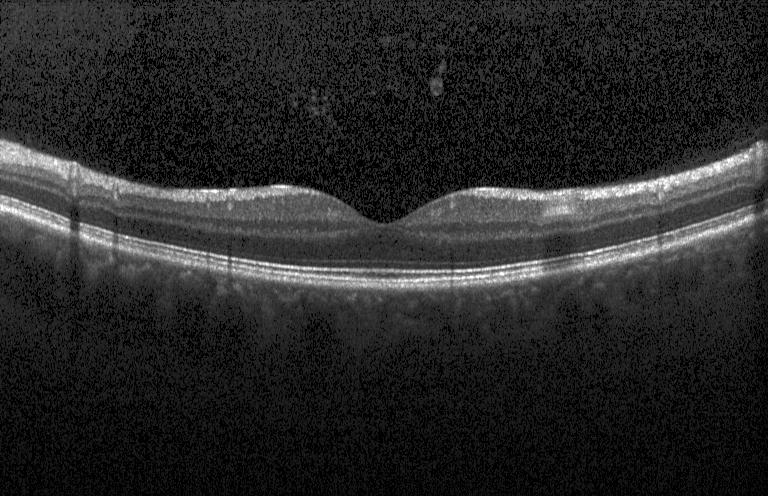 Fovea-centered, spectral-domain OCT, retinal OCT cross-section, Heidelberg Spectralis. Diagnosis: neither choroidal neovascularization, diabetic macular edema, nor drusen.